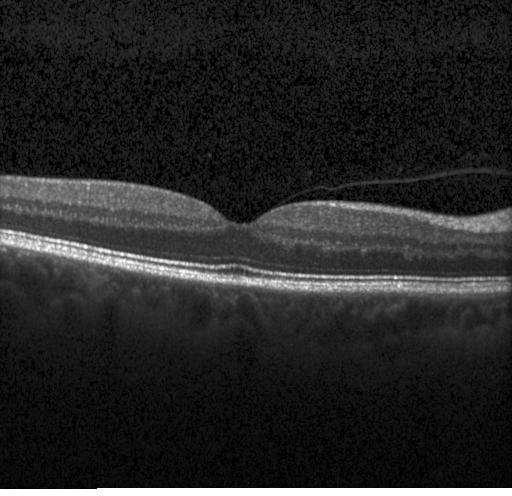 Optical coherence tomography scan, instrument: Heidelberg Spectralis. Impression: no choroidal neovascularization, no diabetic macular edema, and no drusen.